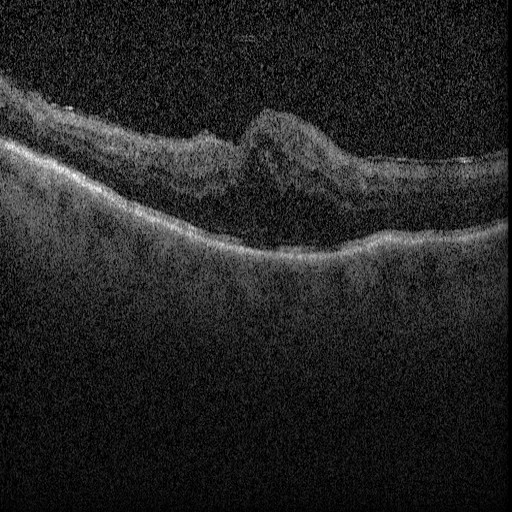 Optical coherence tomography scan. The scan shows diabetic macular edema (DME).